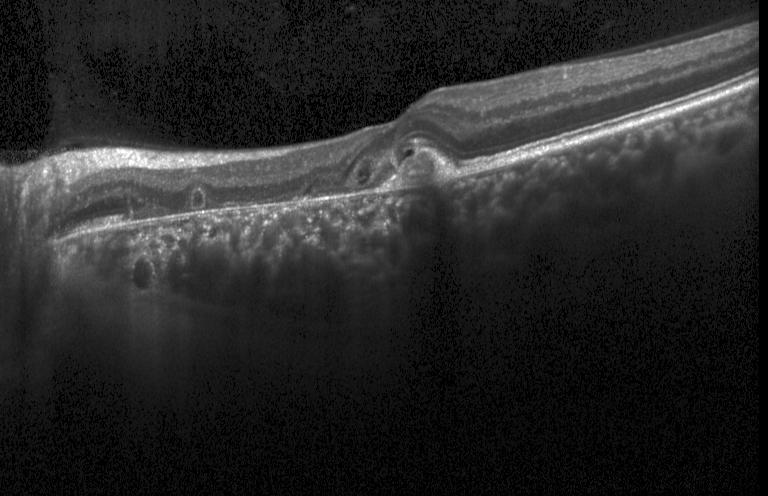

Dx: a choroidal neovascular membrane.